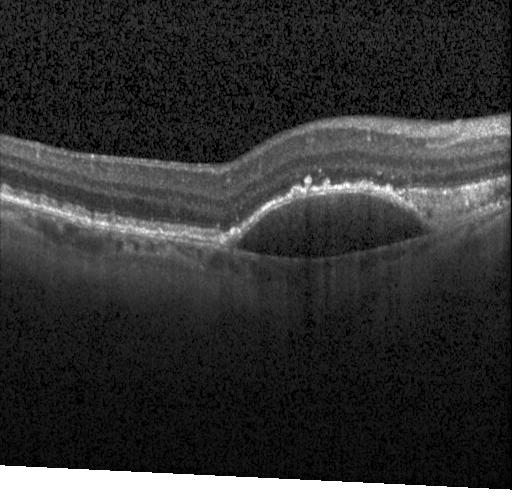

Spectral-domain optical coherence tomography, macular scan, retinal OCT cross-section
Finding: choroidal neovascularization (CNV).